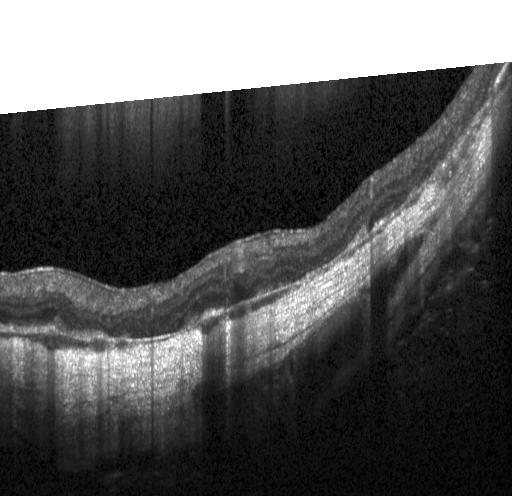

OCT finding: choroidal neovascularization (CNV).